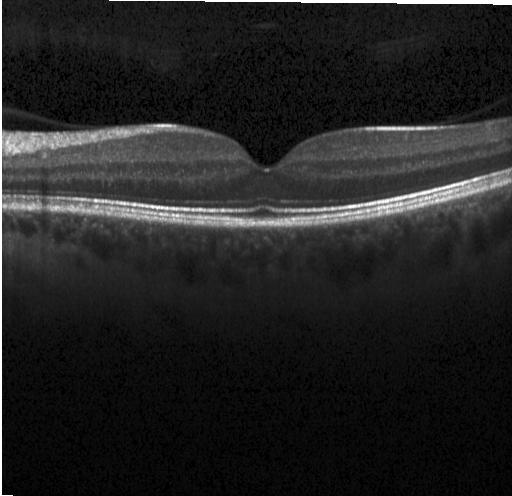 Optical coherence tomography B-scan.
This B-scan demonstrates no evidence of choroidal neovascularization, diabetic macular edema, or drusen.